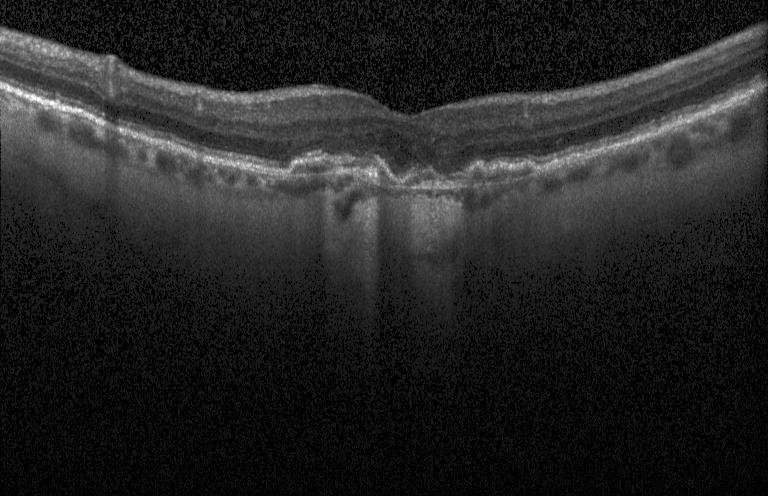 Retinal OCT B-scan, Heidelberg Spectralis
The scan shows a choroidal neovascular membrane.